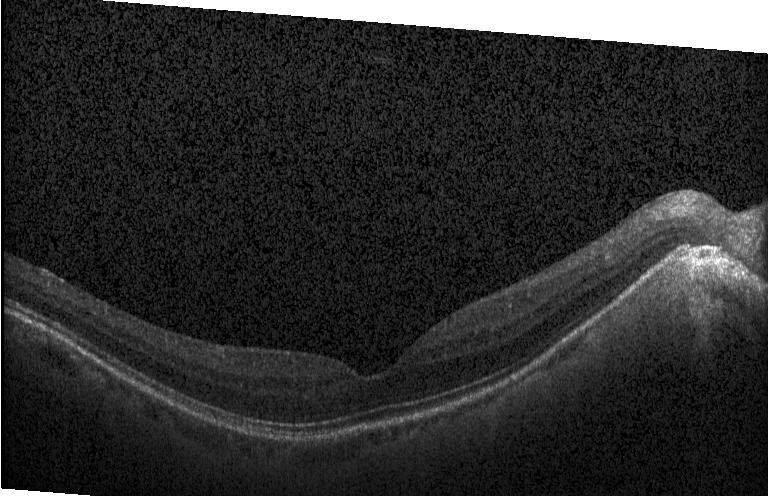

Fovea-centered · acquired on a Heidelberg Spectralis · OCT line scan
Diagnosis: no CNV, DME, or drusen.